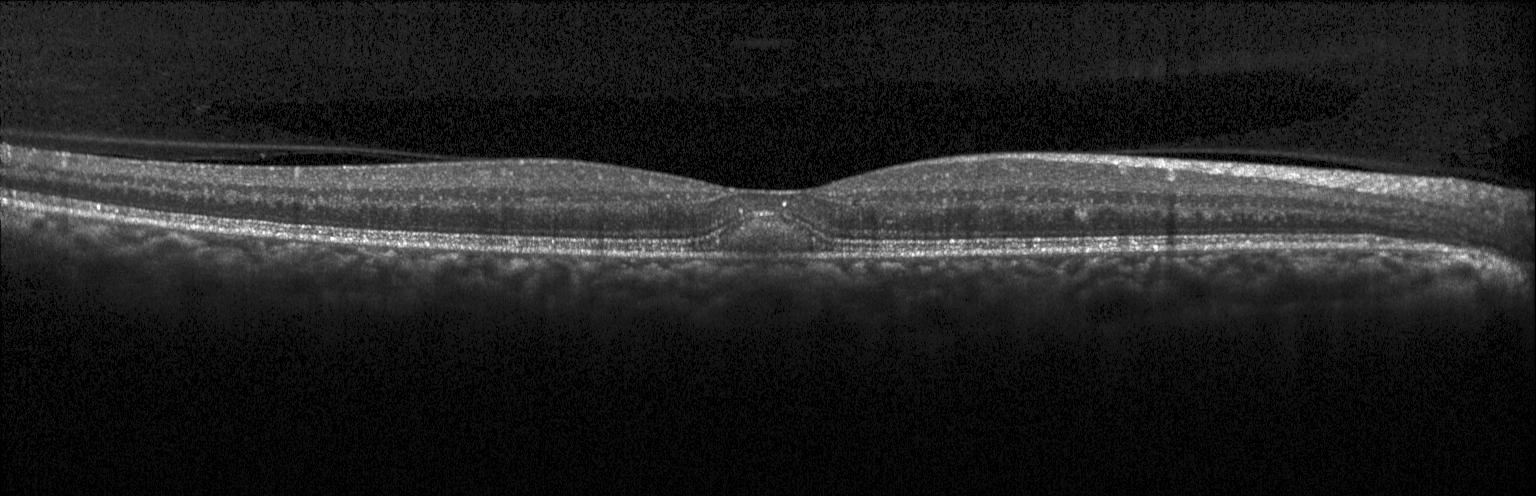

Retinal OCT B-scan
Diagnosis: a choroidal neovascular membrane.